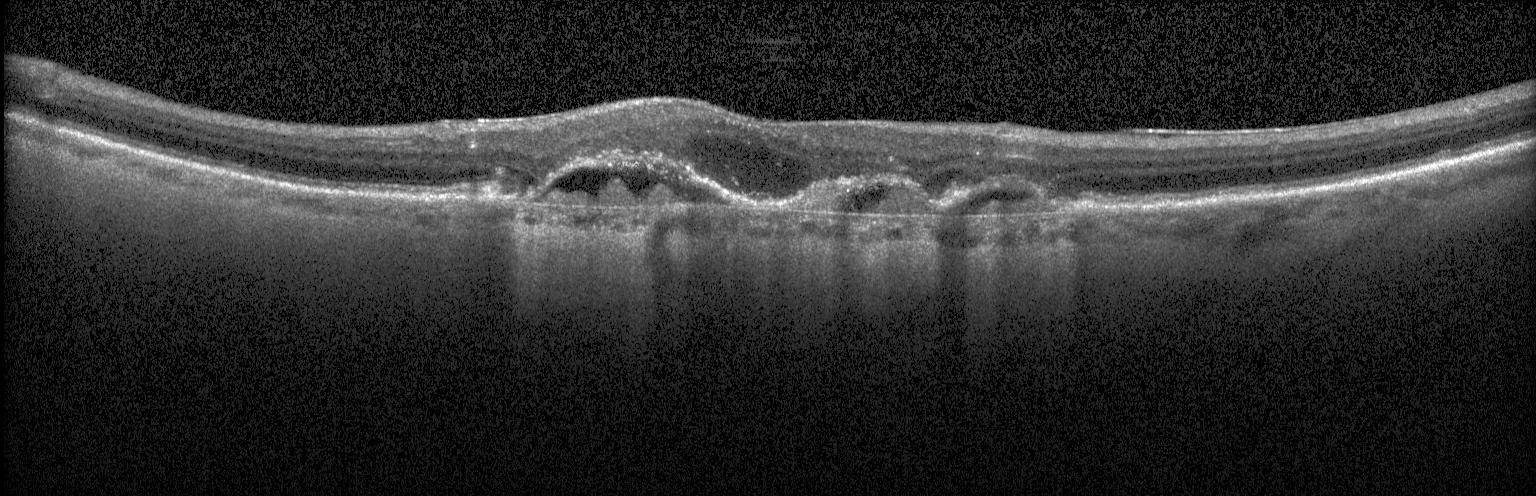 Spectral-domain OCT; Heidelberg Spectralis OCT system; fovea-centered; retinal OCT cross-section — Impression: CNV.